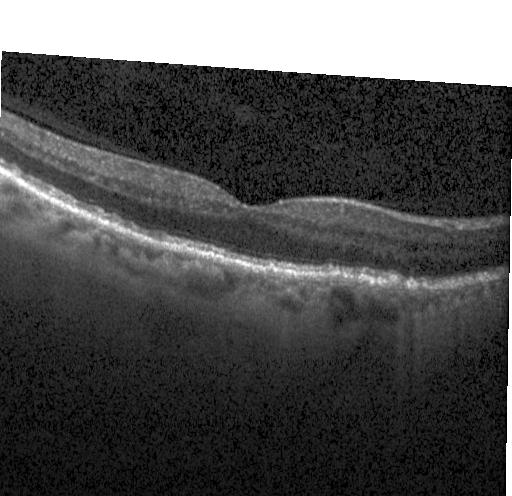 OCT B-scan showing no evidence of choroidal neovascularization, diabetic macular edema, or drusen.